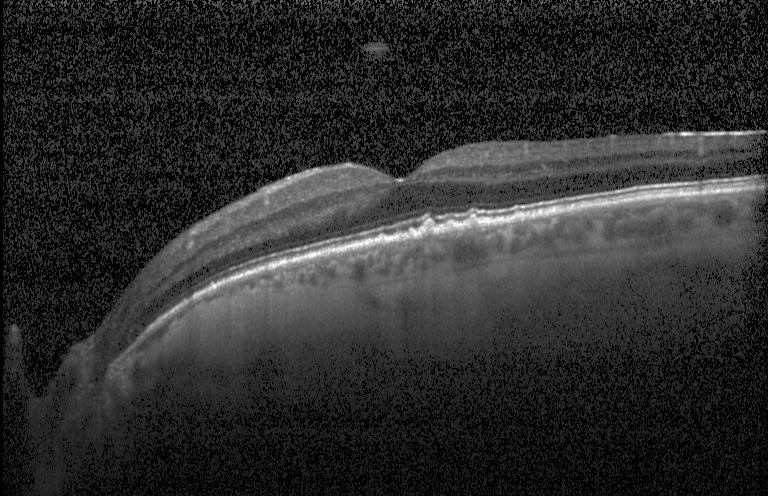 OCT B-scan — The scan shows sub-RPE drusenoid deposits.